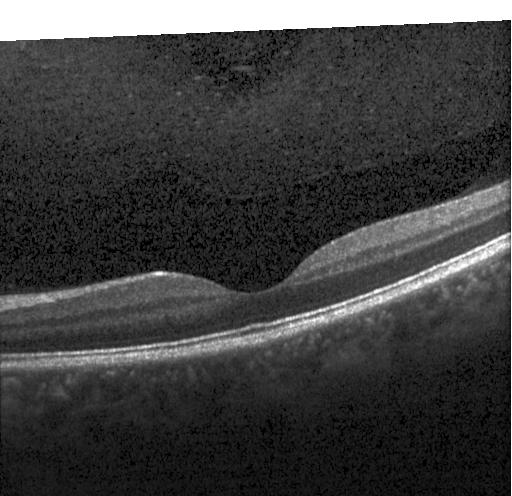
OCT B-scan showing no choroidal neovascularization, diabetic macular edema, or drusen.